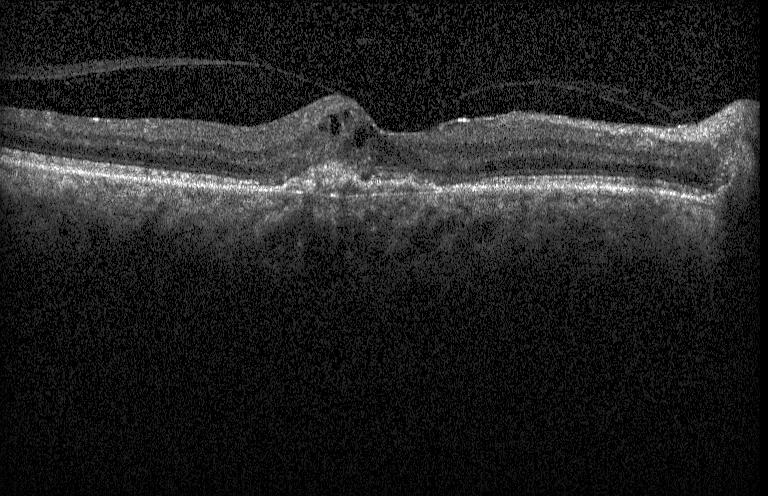

Finding: choroidal neovascularization.